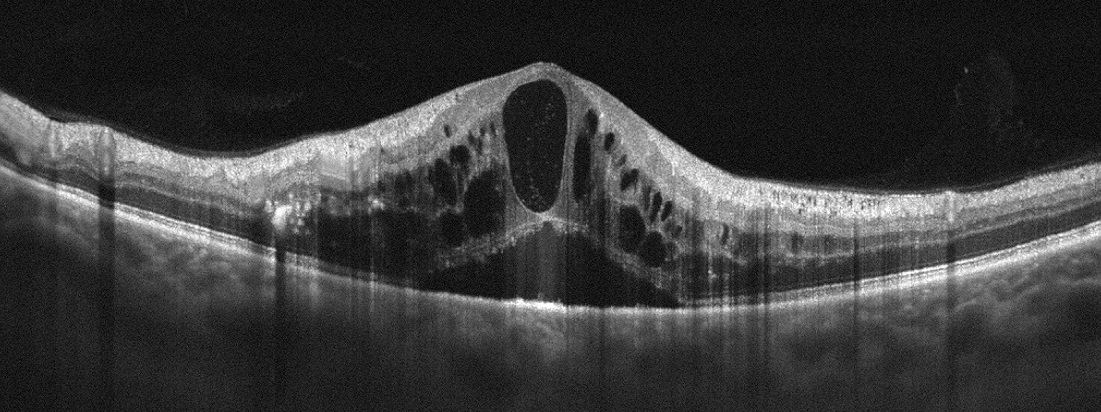
Acquired on an Optovue Avanti RTVue XR. OCT B-scan. Fovea-centered. Diagnosis: retinal vein occlusion (RVO).